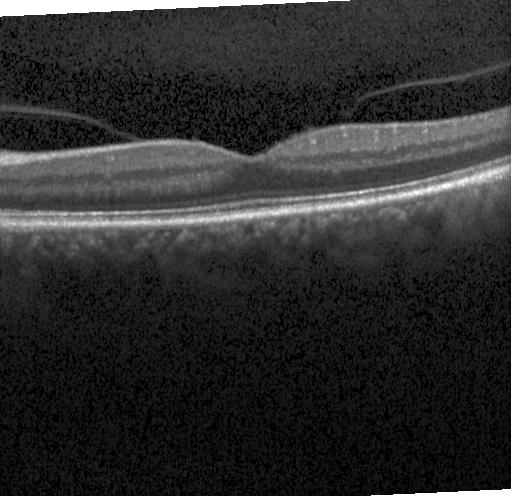

OCT B-scan showing neither choroidal neovascularization, diabetic macular edema, nor drusen.